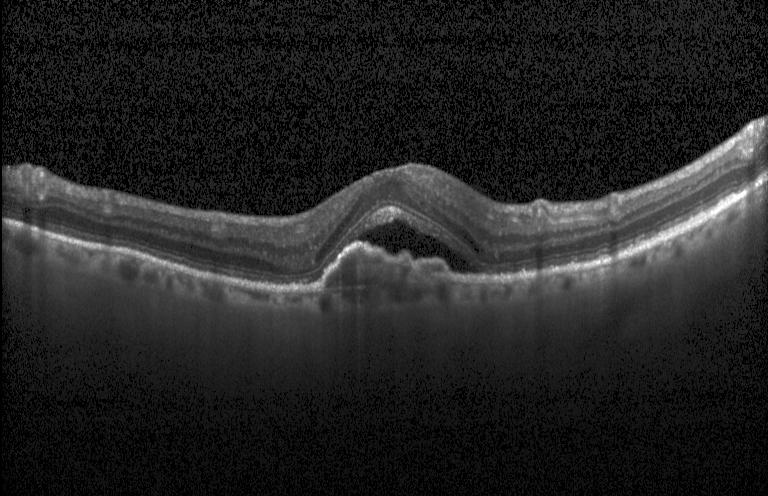
Acquired on a Heidelberg Spectralis, retinal OCT cross-section. Finding: CNV.